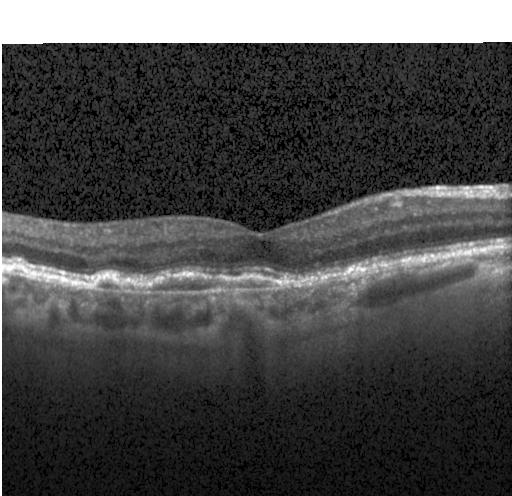 Finding: a choroidal neovascular membrane.